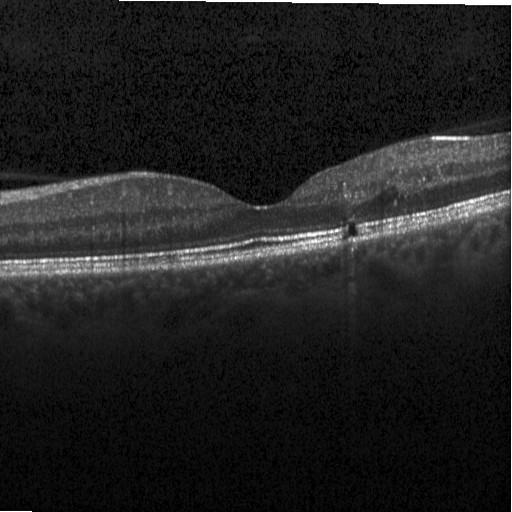
Finding: diabetic macular edema (DME).